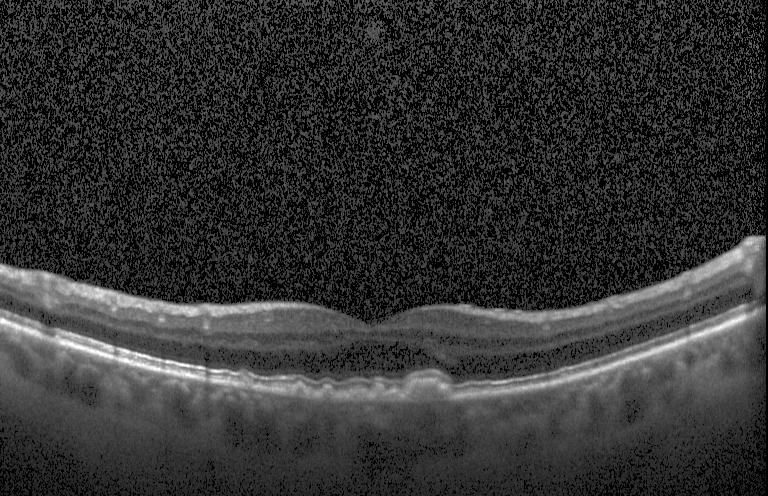

SD-OCT, horizontal scan through the fovea, OCT line scan, Heidelberg Spectralis.
Diagnosis: drusen.